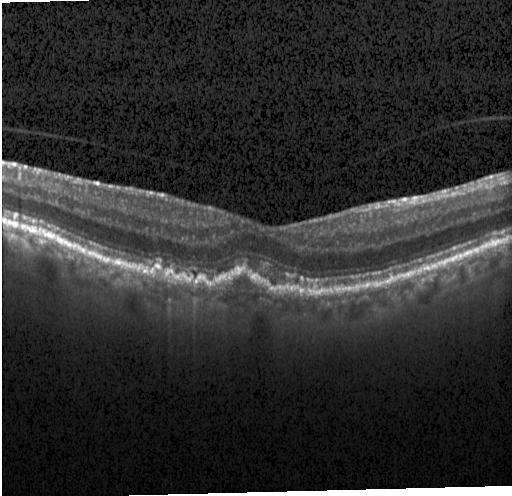
Horizontal scan through the fovea. Retinal OCT cross-section. Finding: choroidal neovascularization.